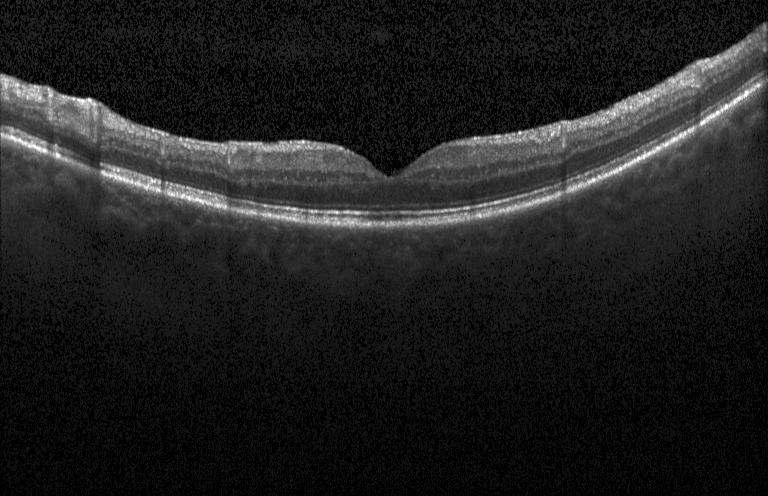
Diagnosis: no choroidal neovascularization, diabetic macular edema, or drusen.